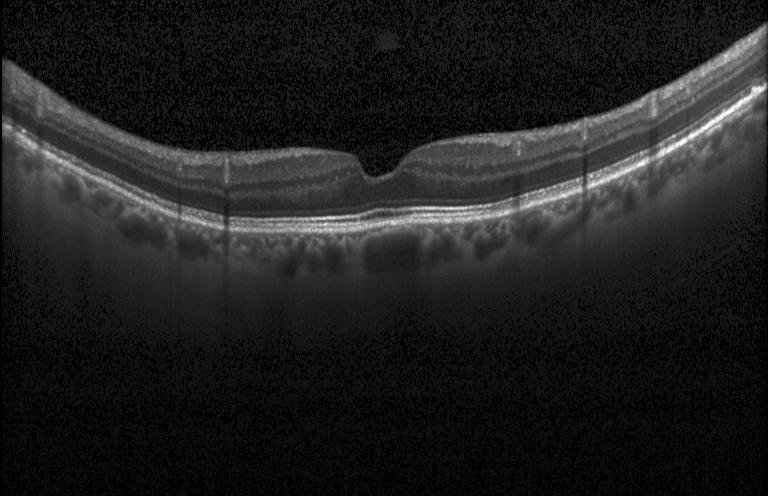 Impression: no evidence of choroidal neovascularization, diabetic macular edema, or drusen.